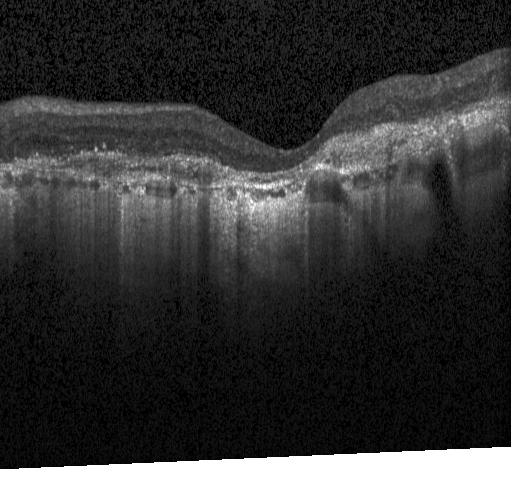 OCT B-scan. Acquired on a Heidelberg Spectralis. Macular scan
This B-scan demonstrates choroidal neovascularization.